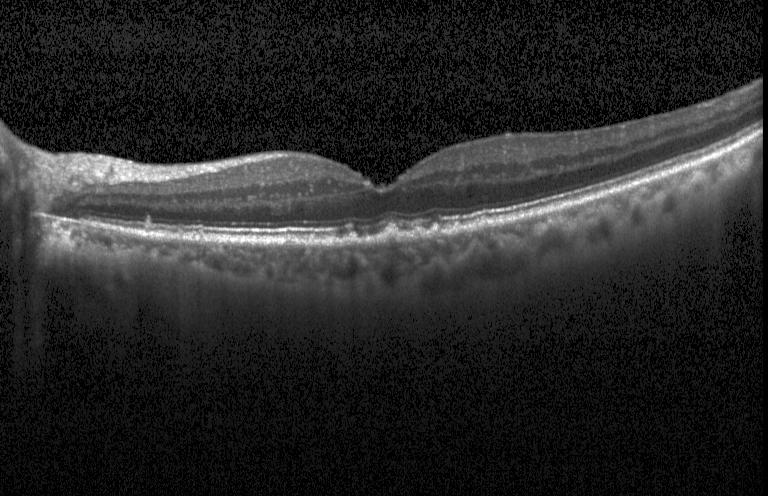 Optical coherence tomography scan; acquired on a Heidelberg Spectralis; SD-OCT. Diagnosis: drusen.